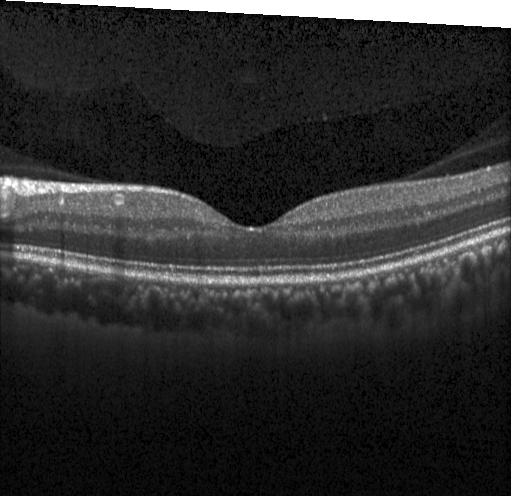
OCT line scan. Acquired on a Heidelberg Spectralis. Spectral-domain optical coherence tomography. Macular scan.
Dx: no CNV, DME, or drusen.